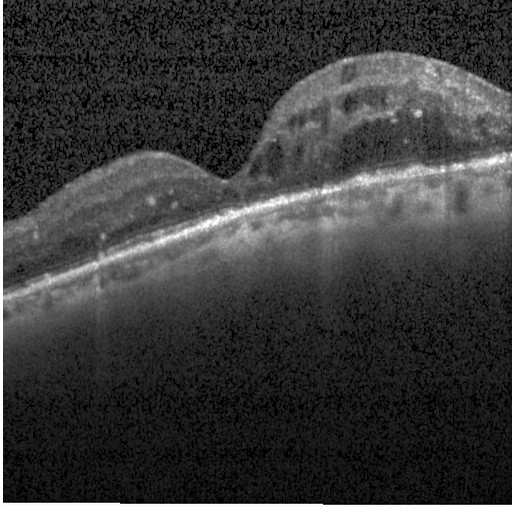 Heidelberg Spectralis OCT system. Optical coherence tomography scan
Finding: DME.